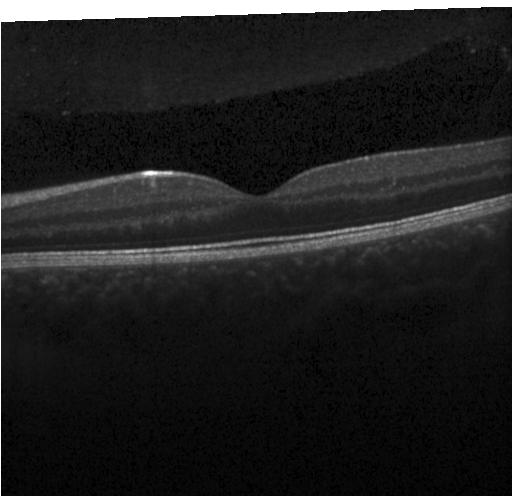 OCT B-scan, centered on the fovea
Impression: no choroidal neovascularization, diabetic macular edema, or drusen.